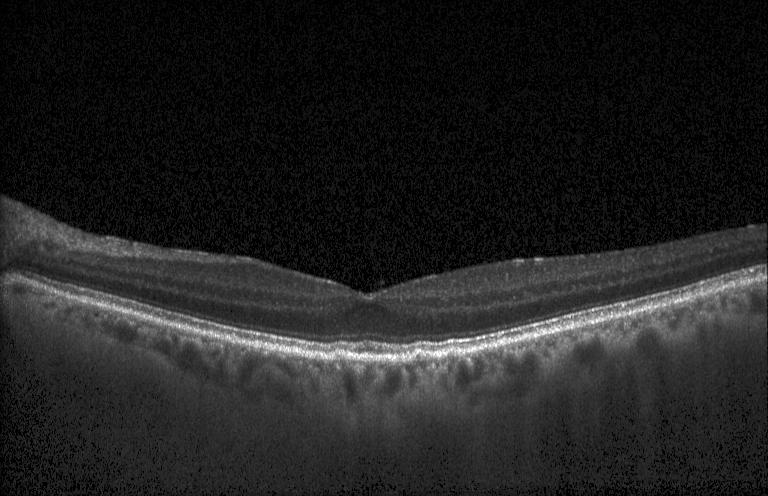
Dx: multiple drusen.